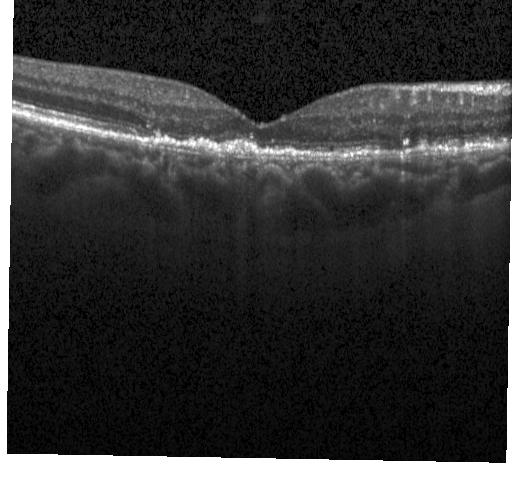 Optical coherence tomography scan. Heidelberg Spectralis OCT system. Centered on the fovea. The scan shows a choroidal neovascular membrane.